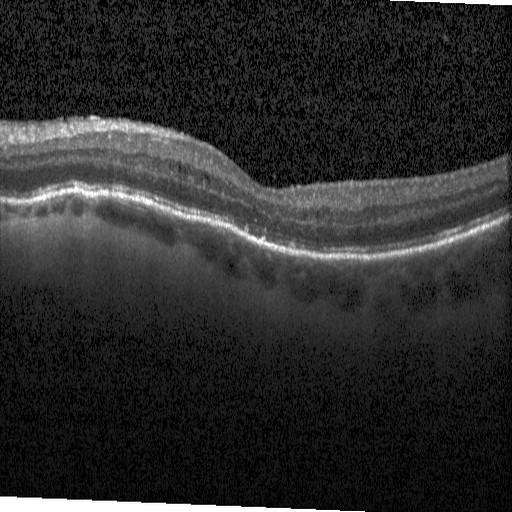

Diagnosis: diabetic macular edema (DME).